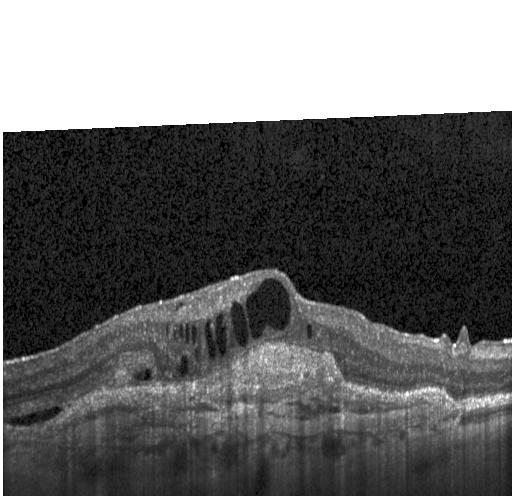

OCT B-scan showing a choroidal neovascular membrane.